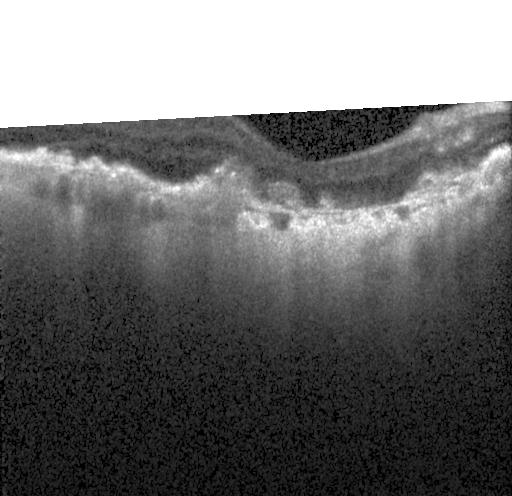 Dx: a choroidal neovascular membrane.